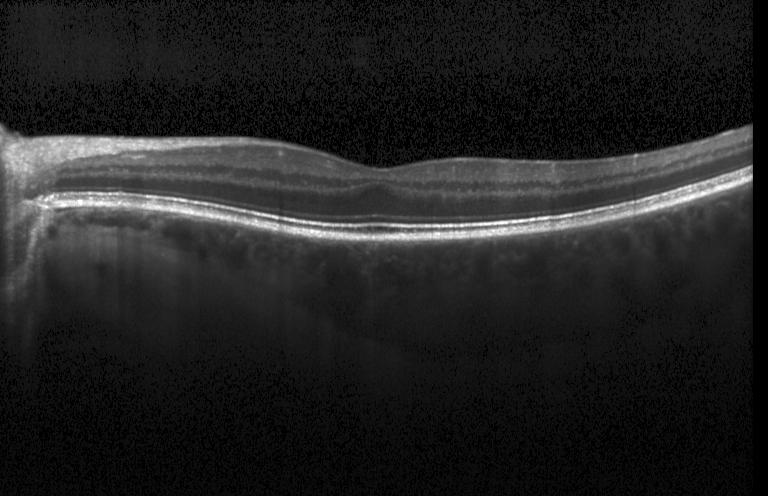

OCT line scan. Macular OCT: no CNV, no DME, and no drusen.